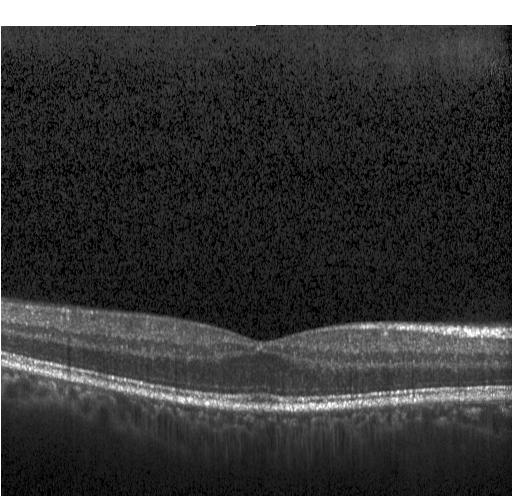

Macular scan, retinal OCT cross-section — OCT finding: no CNV, no DME, and no drusen.